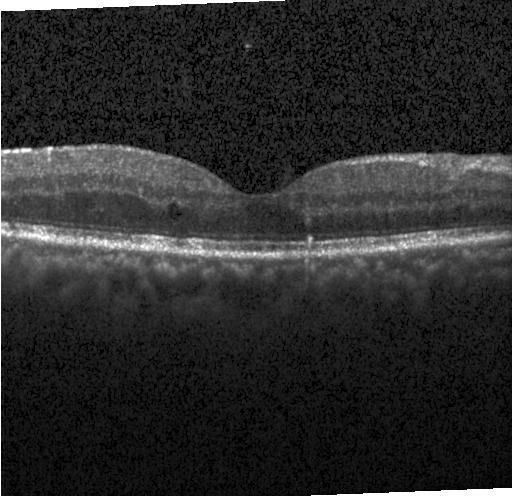
Heidelberg Spectralis OCT system · through the macula · OCT line scan — Impression: diabetic macular edema.